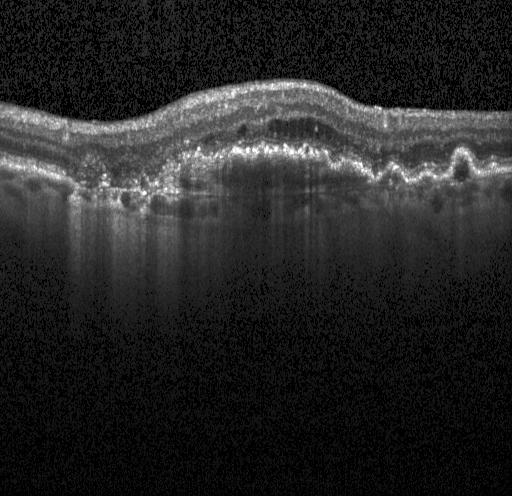 Heidelberg Spectralis OCT system · OCT line scan — Finding: a choroidal neovascular membrane.